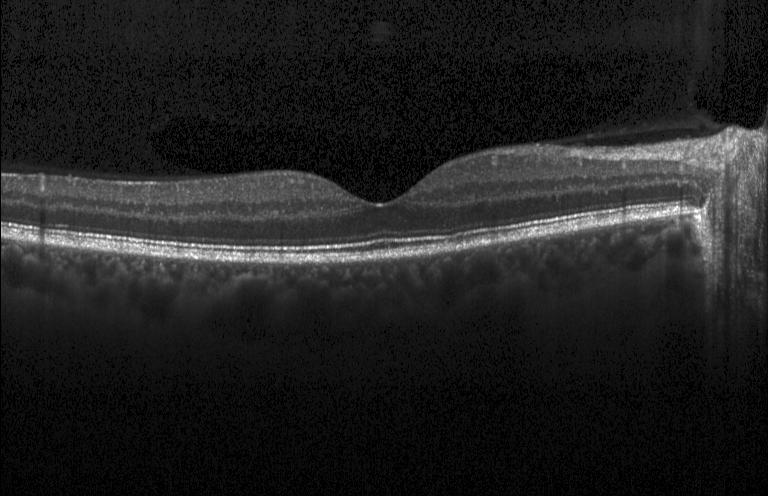

This B-scan demonstrates no choroidal neovascularization, diabetic macular edema, or drusen.